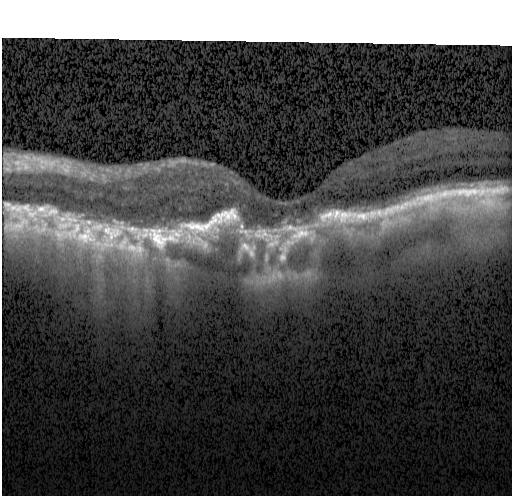 Spectral-domain OCT B-scan: a choroidal neovascular membrane.